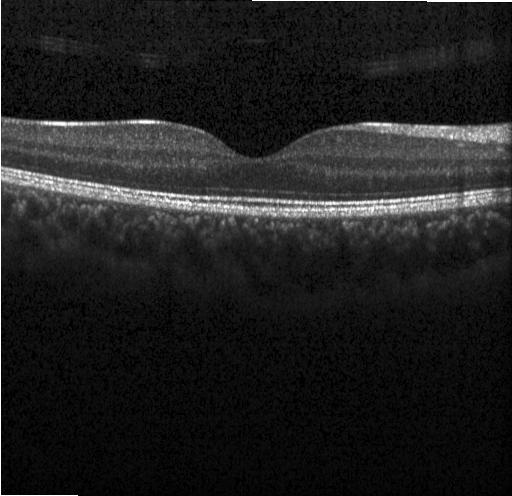

Dx: no evidence of choroidal neovascularization, diabetic macular edema, or drusen.